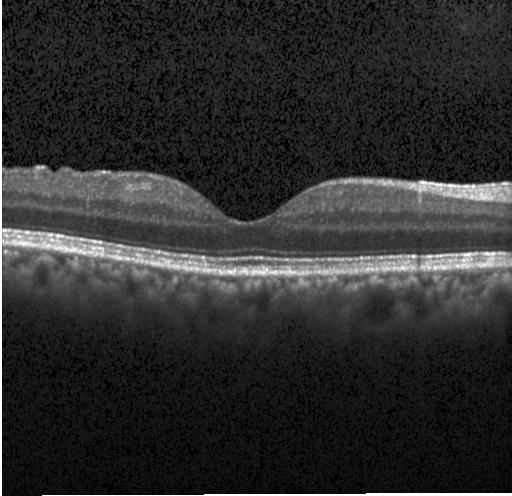

OCT B-scan showing no evidence of CNV, DME, or drusen.